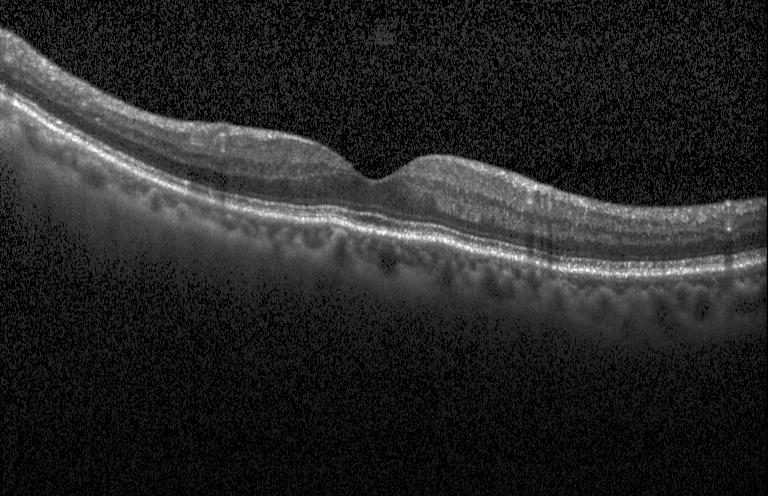 OCT B-scan.
This B-scan demonstrates no choroidal neovascularization, diabetic macular edema, or drusen.